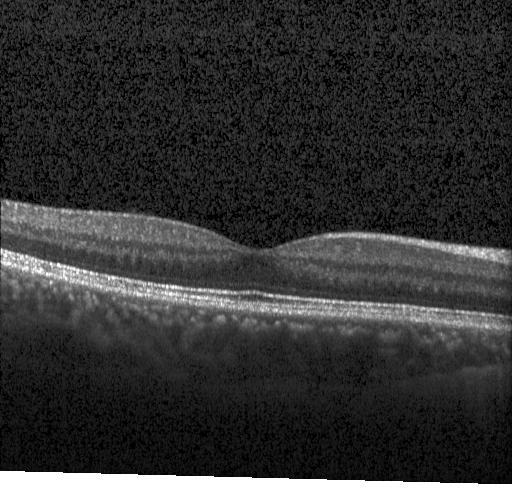
The scan shows no choroidal neovascularization, diabetic macular edema, or drusen.